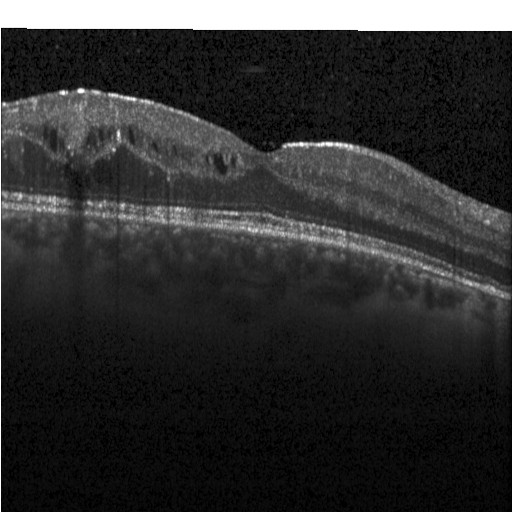

Spectral-domain OCT · macular scan · optical coherence tomography B-scan. Diagnosis: diabetic macular edema (DME).